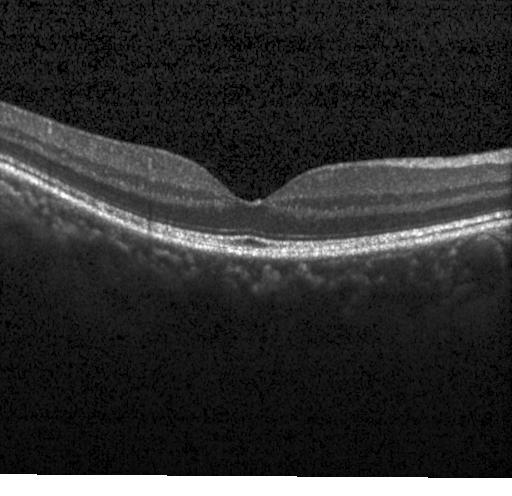

OCT line scan — Diagnosis: no choroidal neovascularization, no diabetic macular edema, and no drusen.